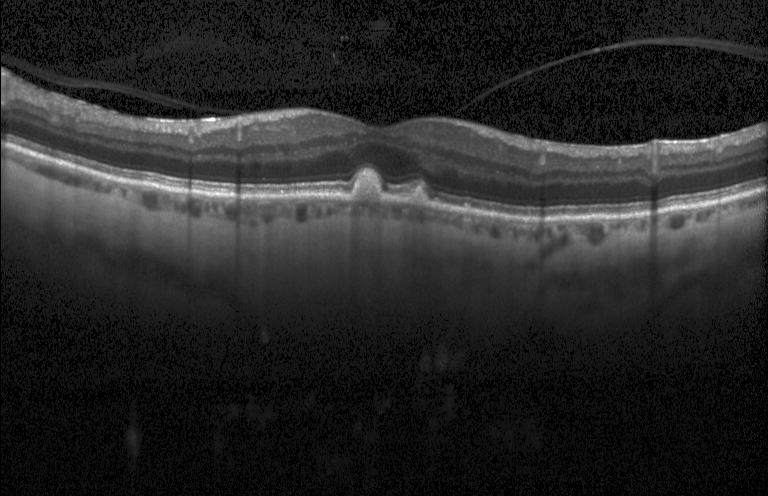
Assessment: sub-RPE drusenoid deposits.